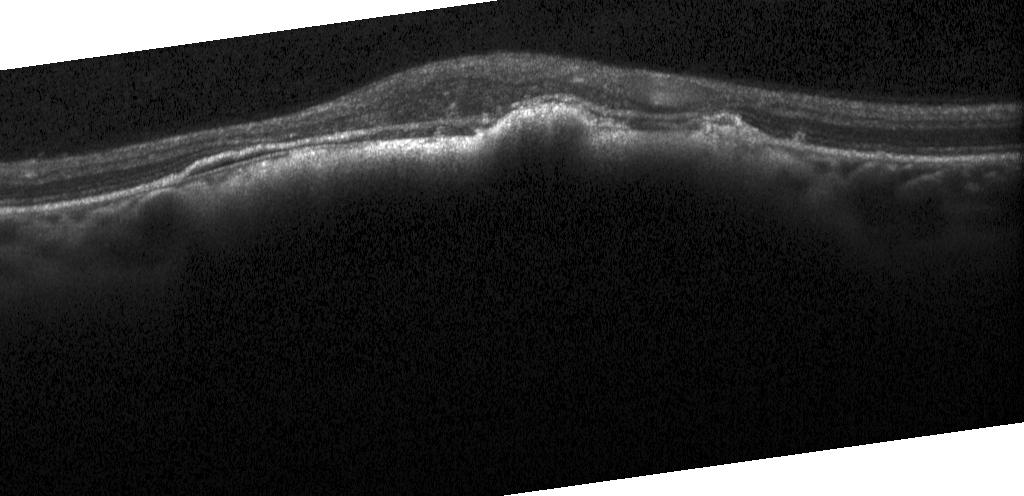

OCT line scan. SD-OCT. Horizontal scan through the fovea
OCT finding: a choroidal neovascular membrane.